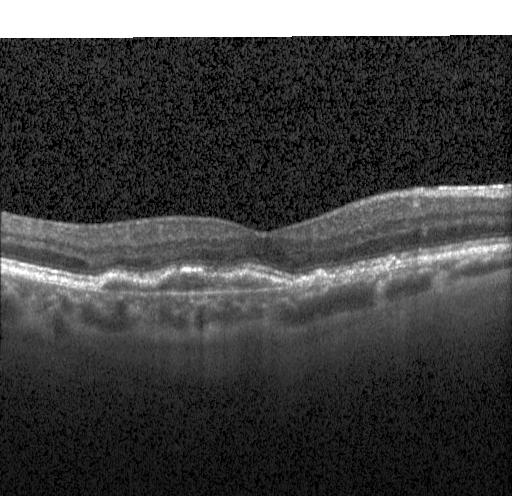

OCT line scan
Finding: a choroidal neovascular membrane.